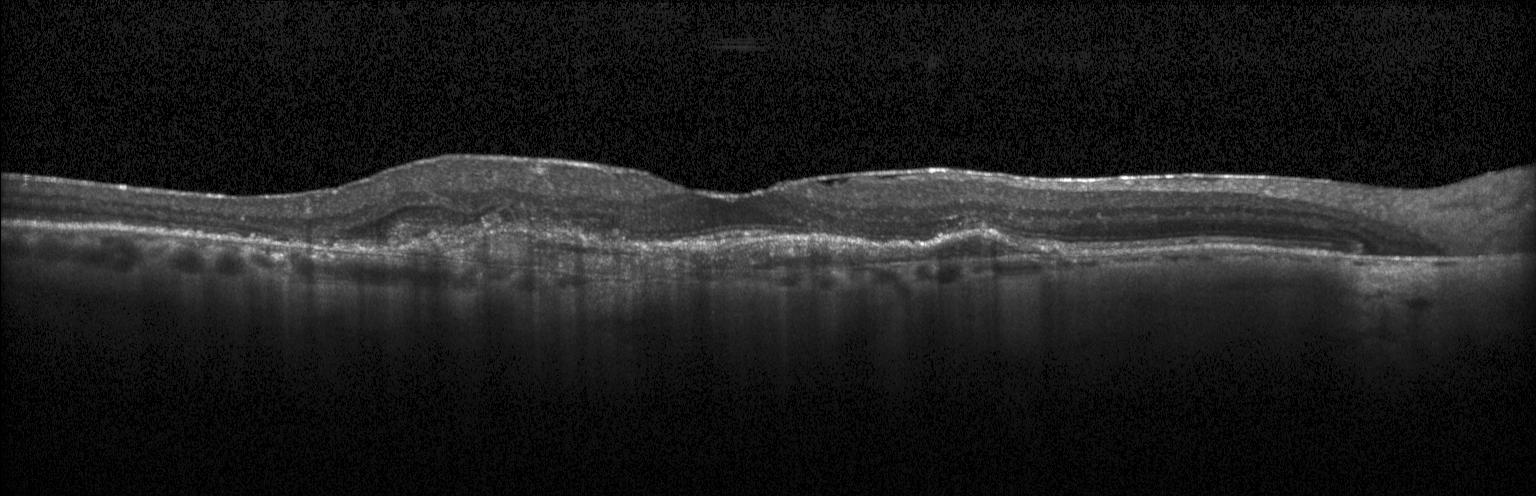

Instrument: Heidelberg Spectralis, optical coherence tomography scan. Assessment: a choroidal neovascular membrane.